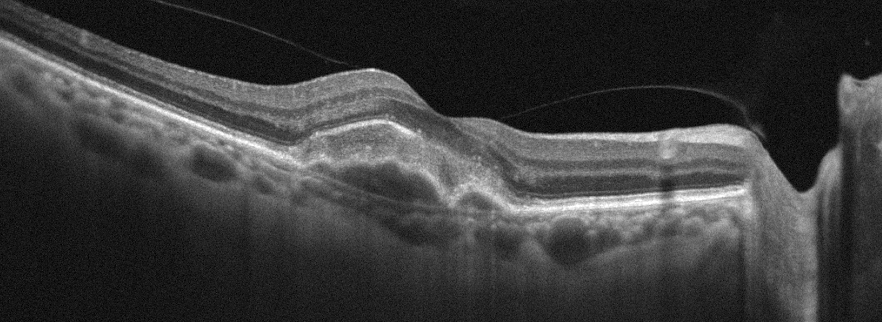
Right eye. Retinal OCT B-scan.
Dx: age-related macular degeneration.